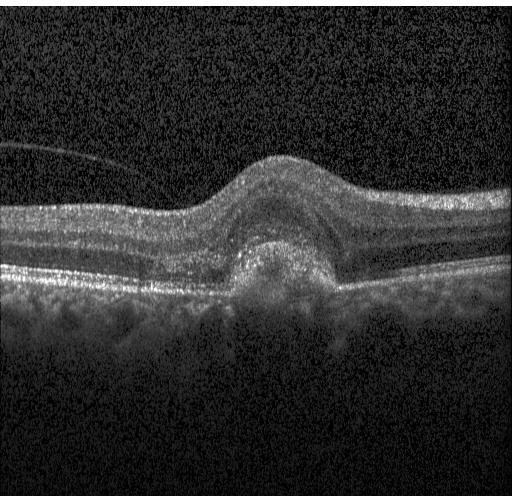 Retinal OCT B-scan
Finding: a choroidal neovascular membrane.